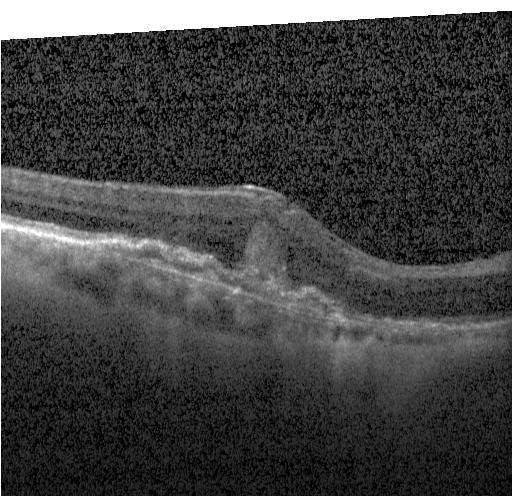

Diagnosis: choroidal neovascularization (CNV).